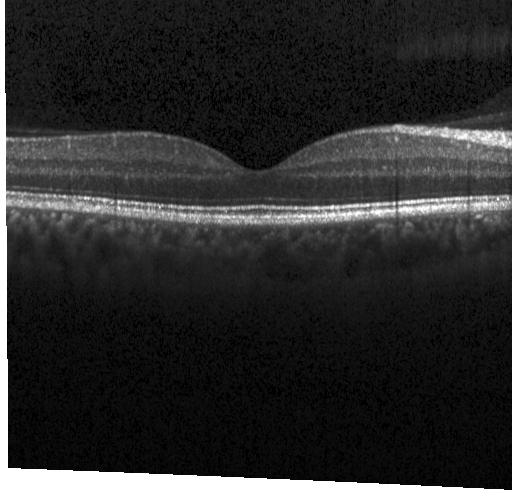
SD-OCT; Heidelberg Spectralis; macular scan; OCT line scan. Finding: no choroidal neovascularization, no diabetic macular edema, and no drusen.